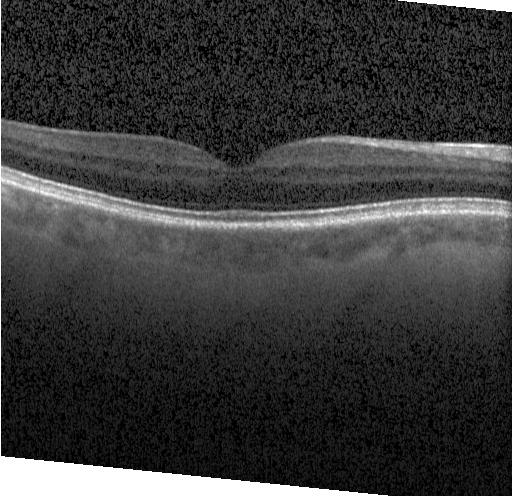 Diagnosis: neither CNV, DME, nor drusen.